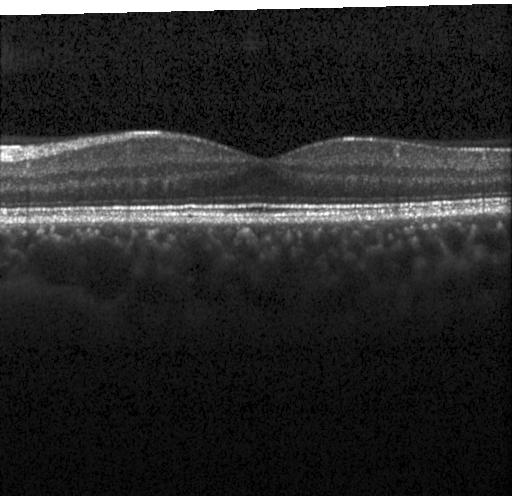

Acquired on a Heidelberg Spectralis; retinal OCT cross-section.
Macular OCT: neither CNV, DME, nor drusen.